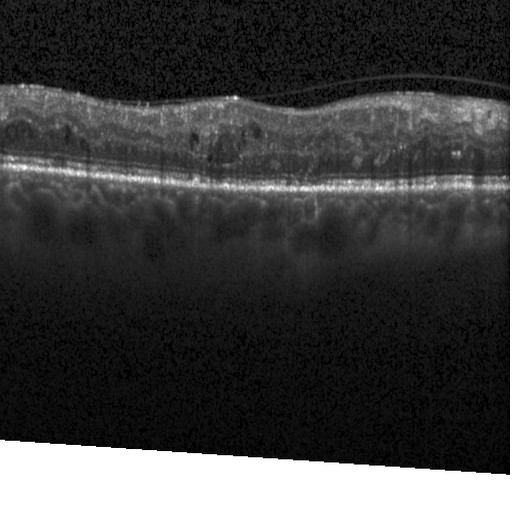 Impression: diabetic macular edema (DME).